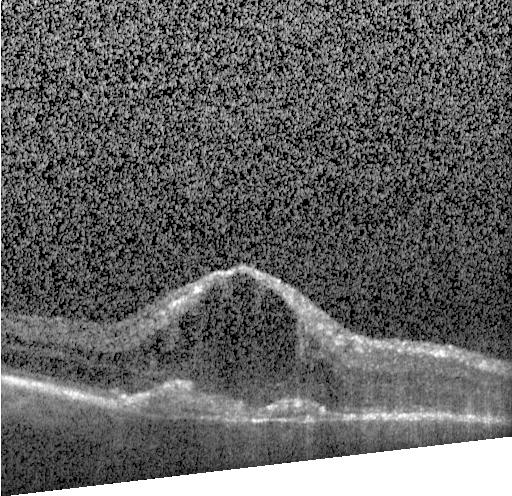 Retinal OCT B-scan.
Impression: choroidal neovascularization (CNV).